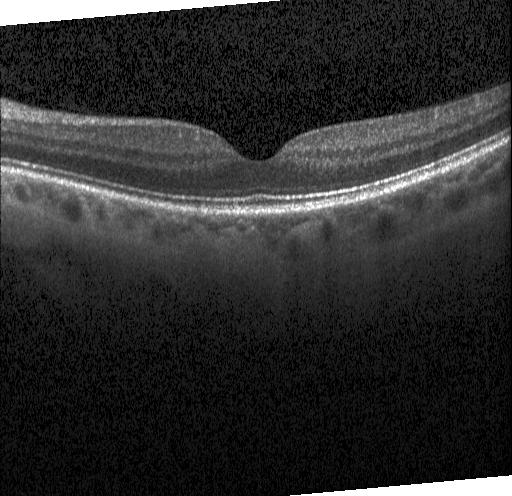 Spectral-domain OCT. Retinal OCT B-scan
OCT finding: no choroidal neovascularization, diabetic macular edema, or drusen.